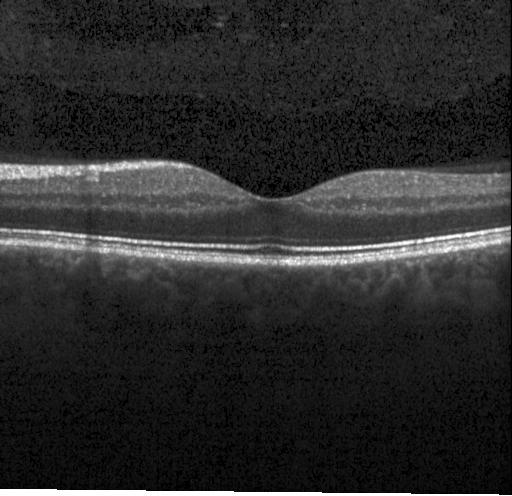

SD-OCT. Retinal OCT B-scan. Fovea-centered. Heidelberg Spectralis.
Diagnosis: no CNV, no DME, and no drusen.